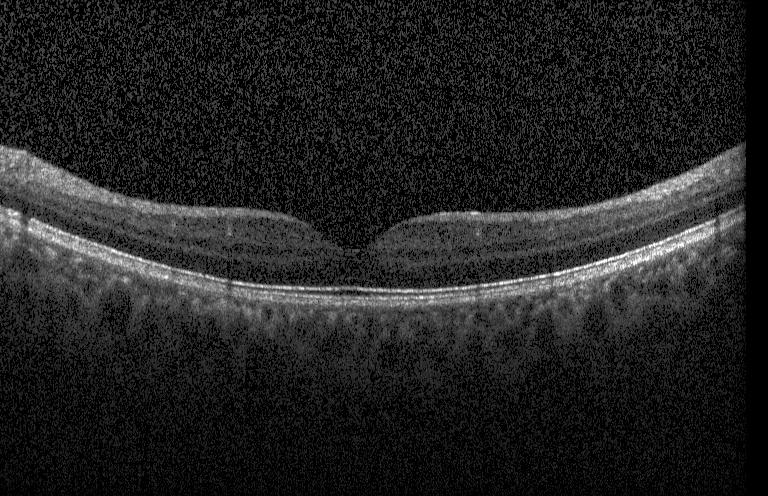

Diagnosis: no choroidal neovascularization, diabetic macular edema, or drusen.